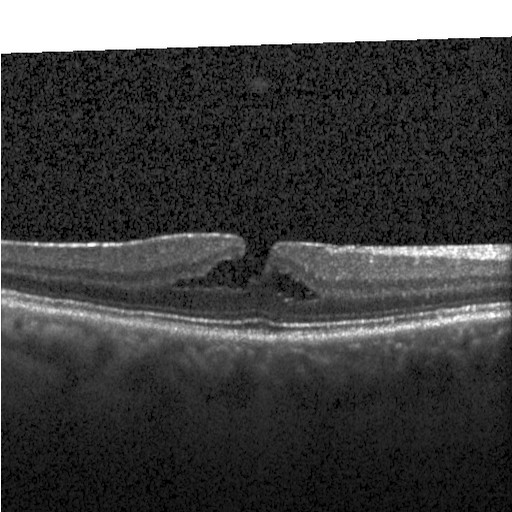
Instrument: Heidelberg Spectralis · macular scan · optical coherence tomography B-scan · SD-OCT — Diagnosis: diabetic macular edema (DME).